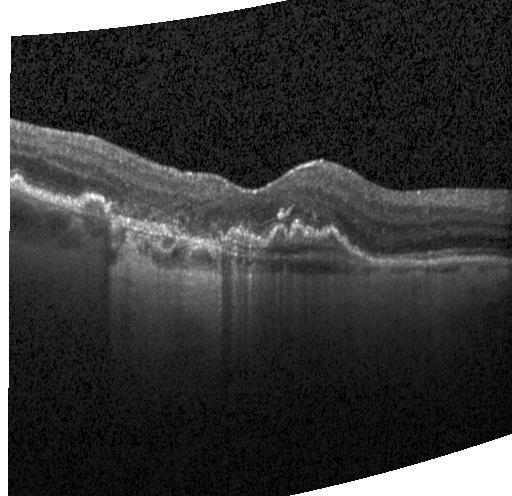 Spectral-domain optical coherence tomography, Heidelberg Spectralis, OCT B-scan, macular scan. Assessment: a choroidal neovascular membrane.